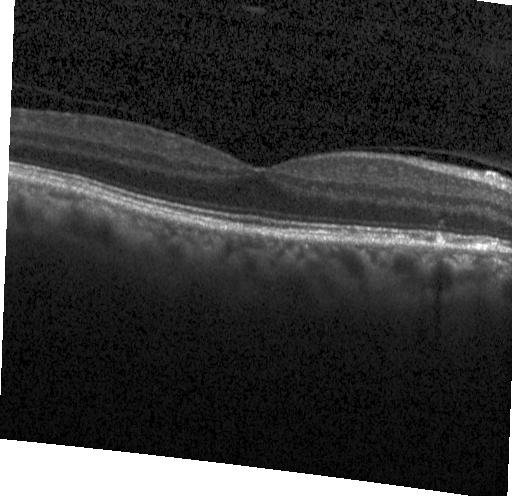 OCT line scan. Instrument: Heidelberg Spectralis
This B-scan demonstrates multiple drusen.